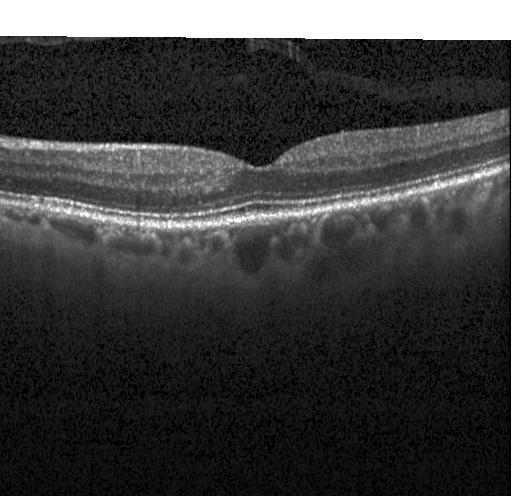 OCT B-scan, acquired on a Heidelberg Spectralis
Macular OCT: neither choroidal neovascularization, diabetic macular edema, nor drusen.